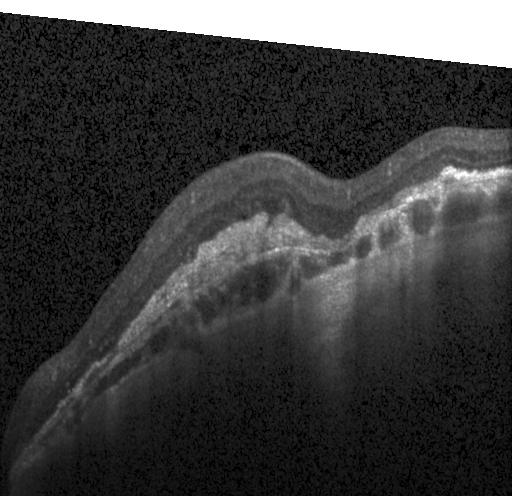
Centered on the fovea · spectral-domain OCT · optical coherence tomography B-scan
Diagnosis: CNV.